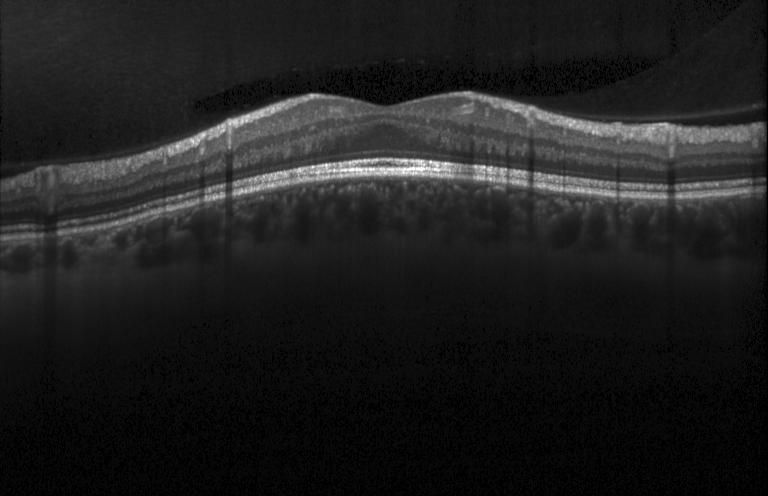 Heidelberg Spectralis OCT system. OCT B-scan — Finding: no choroidal neovascularization, no diabetic macular edema, and no drusen.